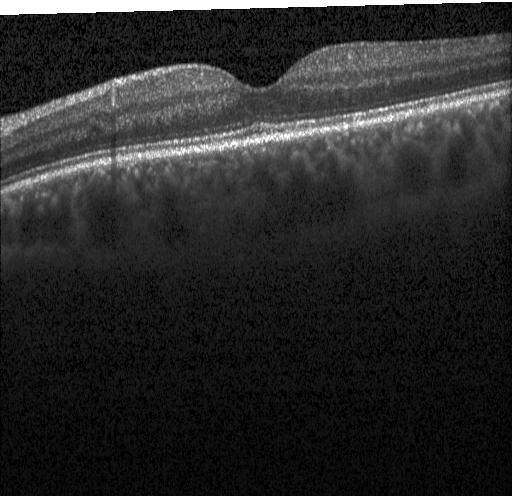 Retinal OCT B-scan. No choroidal neovascularization, diabetic macular edema, or drusen.